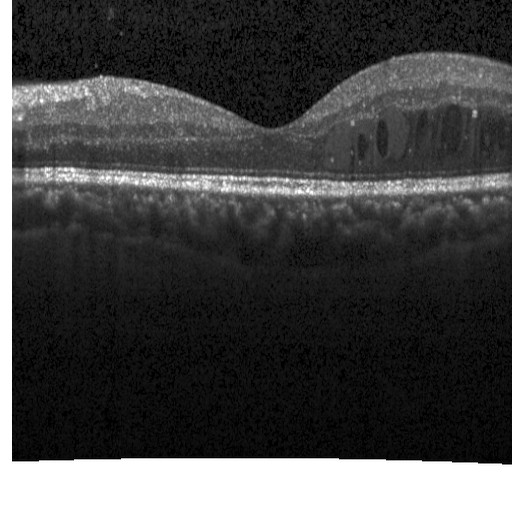

Horizontal scan through the fovea · OCT B-scan. Macular OCT: diabetic macular edema (DME).